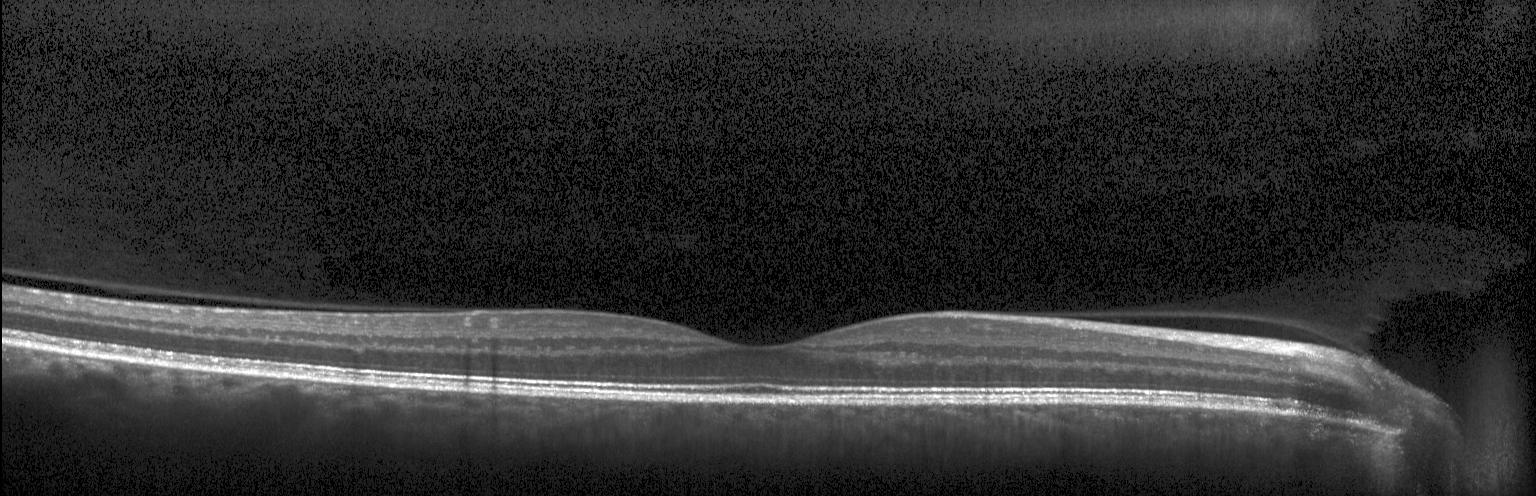

Spectral-domain optical coherence tomography; OCT B-scan.
The scan shows neither choroidal neovascularization, diabetic macular edema, nor drusen.